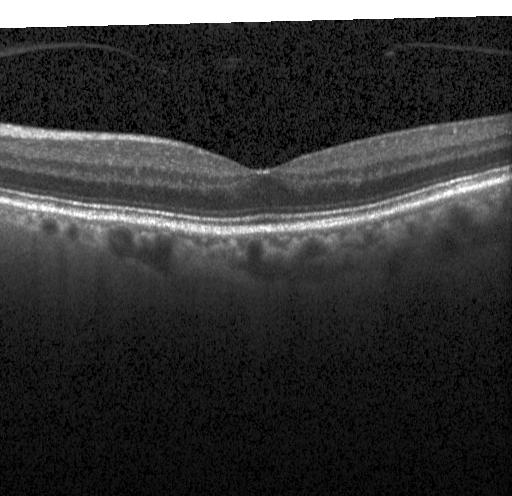
Impression: no evidence of choroidal neovascularization, diabetic macular edema, or drusen.